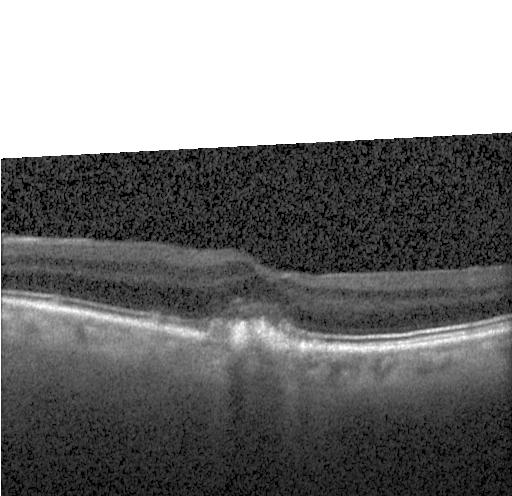

OCT B-scan, instrument: Heidelberg Spectralis
Diagnosis: choroidal neovascularization (CNV).